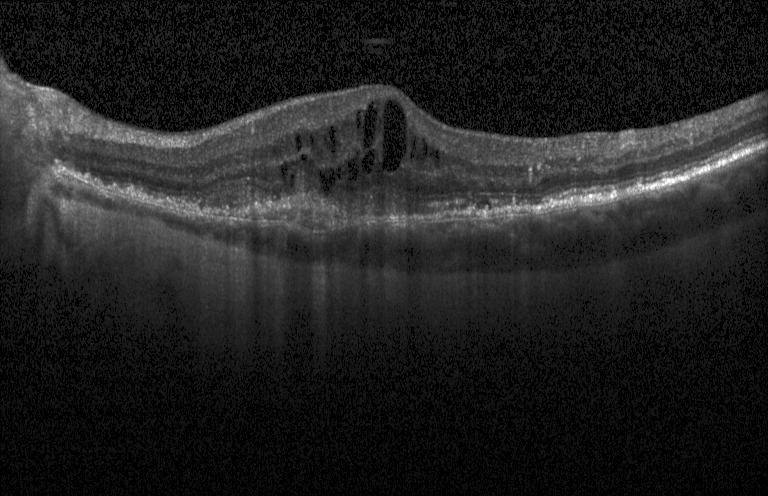
Impression: a choroidal neovascular membrane.